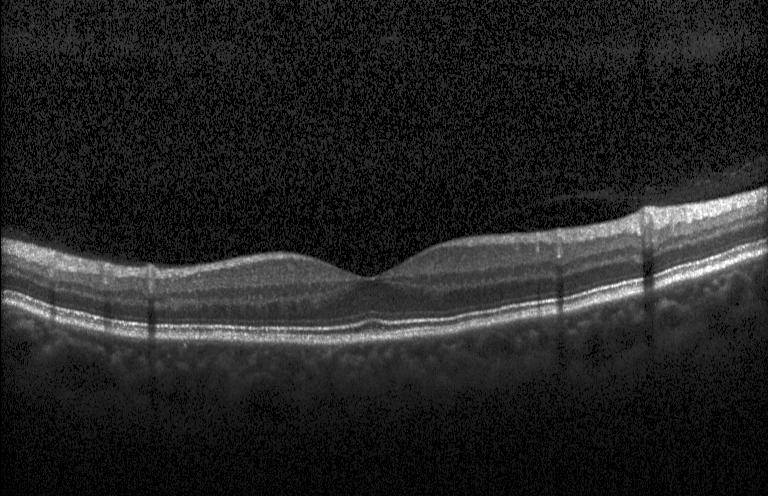
OCT line scan · SD-OCT.
Impression: no evidence of choroidal neovascularization, diabetic macular edema, or drusen.